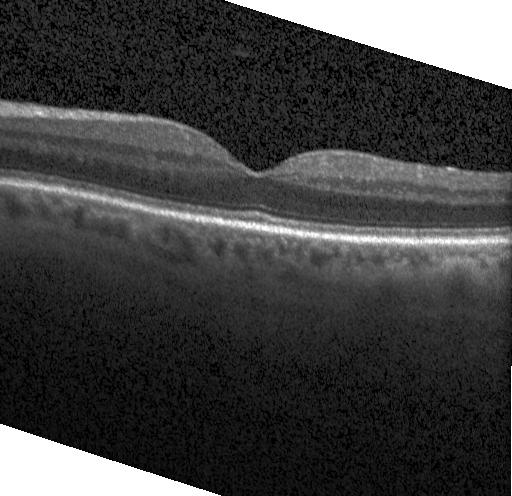

OCT line scan — No choroidal neovascularization, no diabetic macular edema, and no drusen.